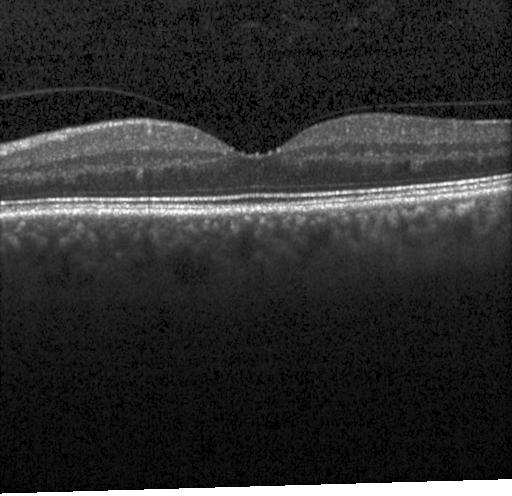

Diagnosis: no CNV, DME, or drusen.